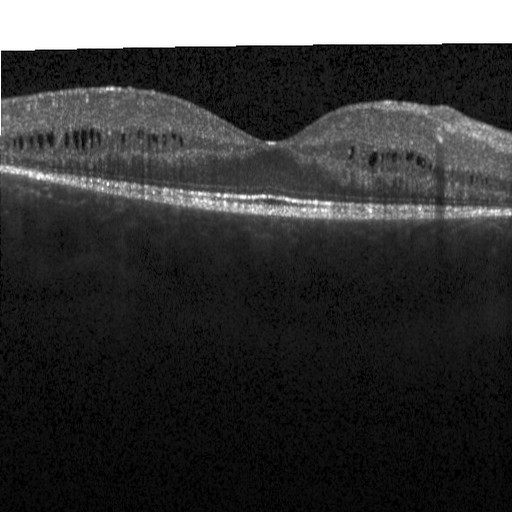
DME.